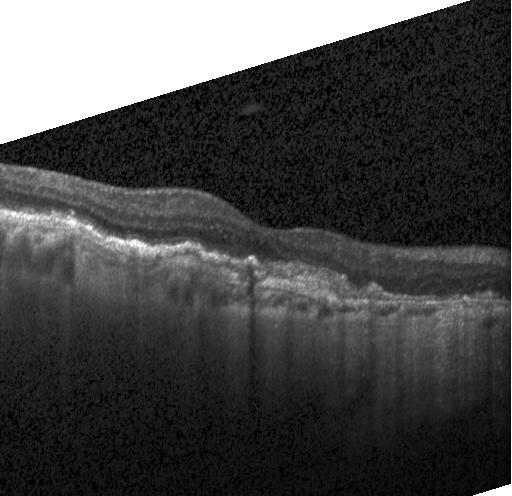

Spectral-domain OCT. Retinal OCT B-scan. Heidelberg Spectralis. Macular scan. OCT finding: a choroidal neovascular membrane.